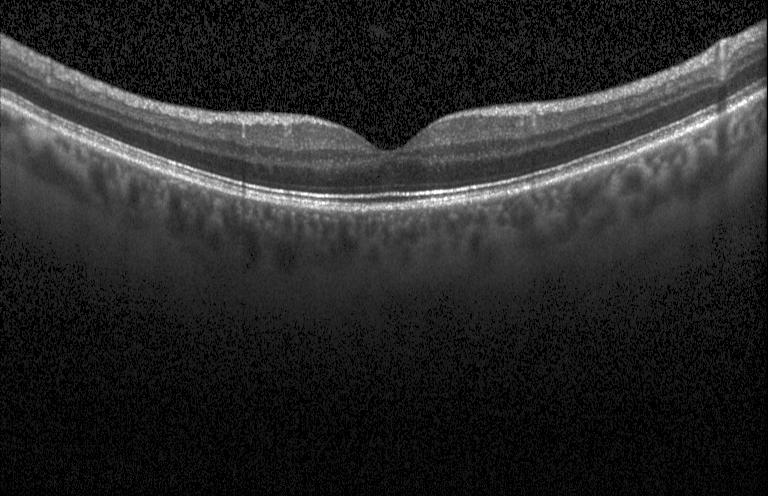 Spectral-domain OCT · retinal OCT B-scan · acquired on a Heidelberg Spectralis · macular scan. Finding: neither choroidal neovascularization, diabetic macular edema, nor drusen.